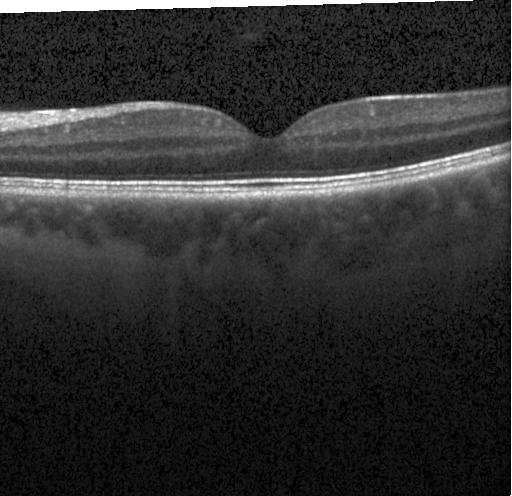
Diagnosis: no CNV, DME, or drusen.